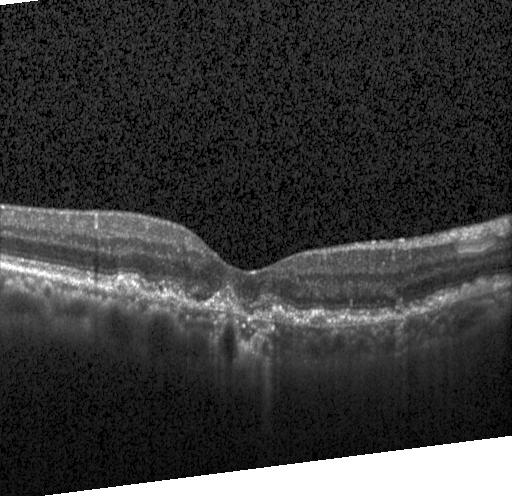

Finding: CNV.